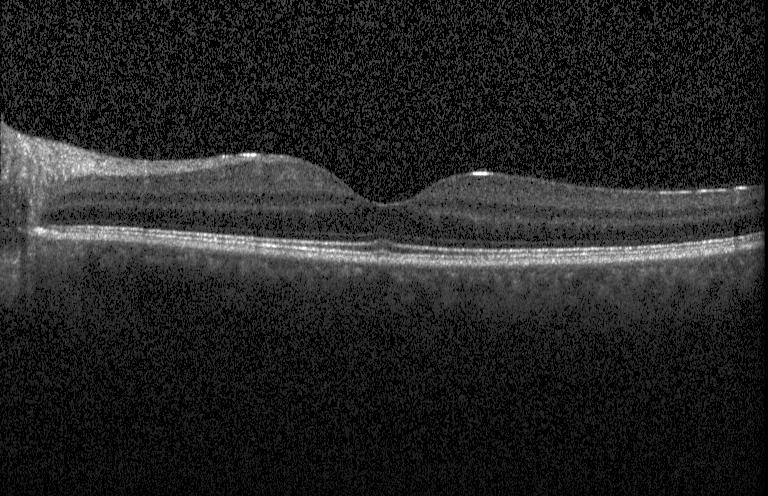
Impression: no evidence of choroidal neovascularization, diabetic macular edema, or drusen.